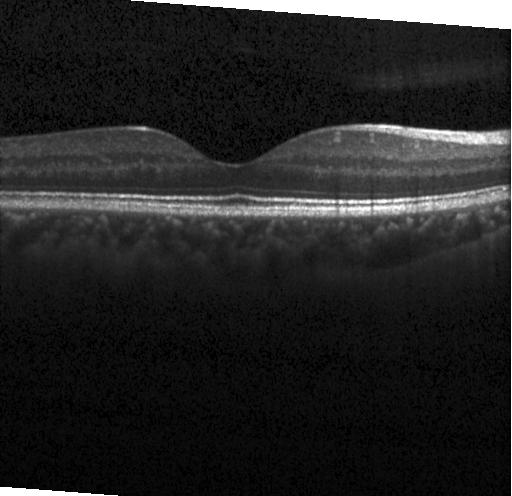

Optical coherence tomography scan — This B-scan demonstrates no evidence of choroidal neovascularization, diabetic macular edema, or drusen.